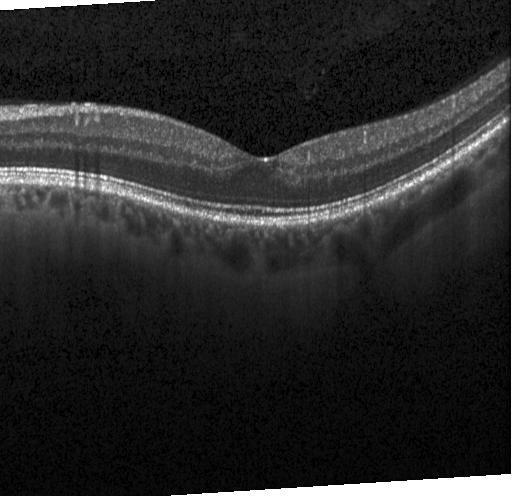 Retinal OCT cross-section showing neither choroidal neovascularization, diabetic macular edema, nor drusen.